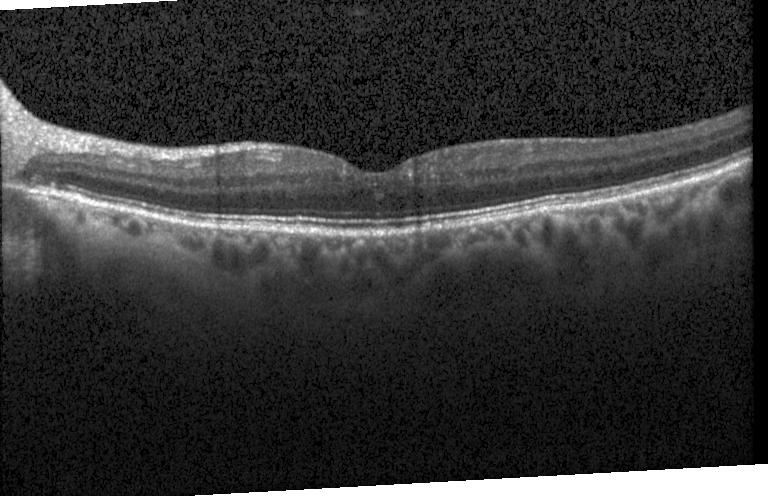

OCT scan showing no choroidal neovascularization, no diabetic macular edema, and no drusen.